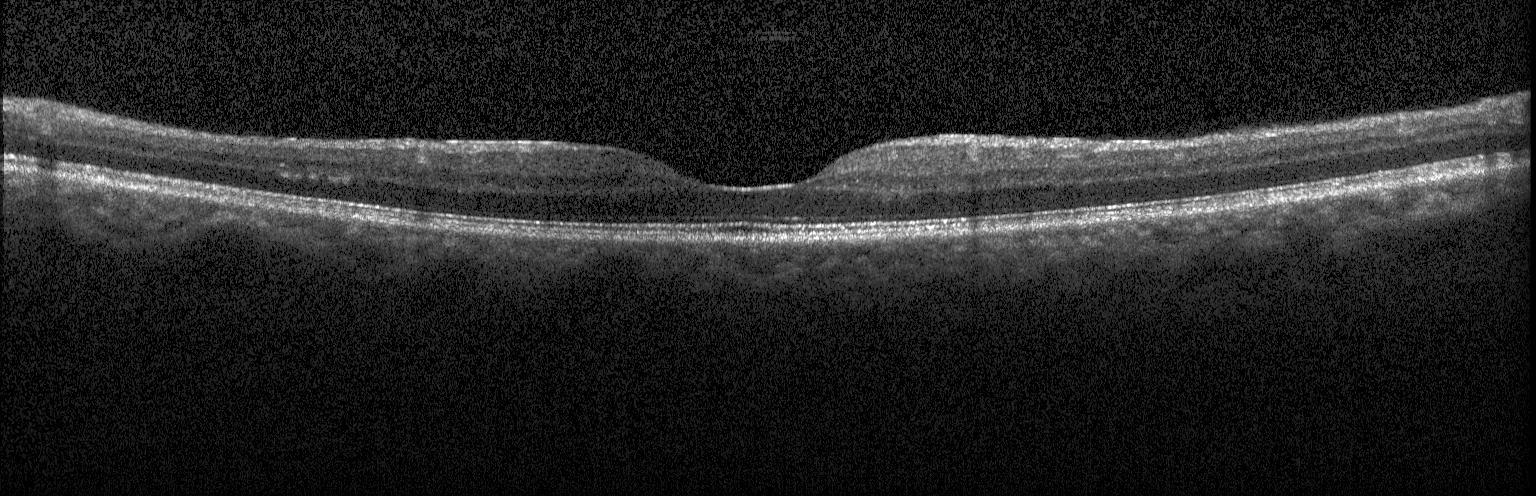 Macular scan. Retinal OCT cross-section. Diagnosis: neither CNV, DME, nor drusen.